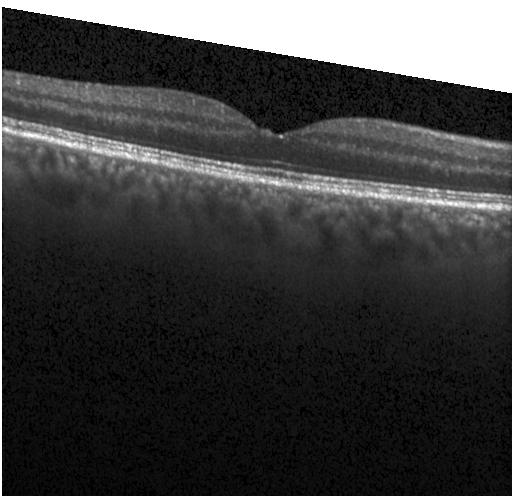

Diagnosis: no choroidal neovascularization, no diabetic macular edema, and no drusen.